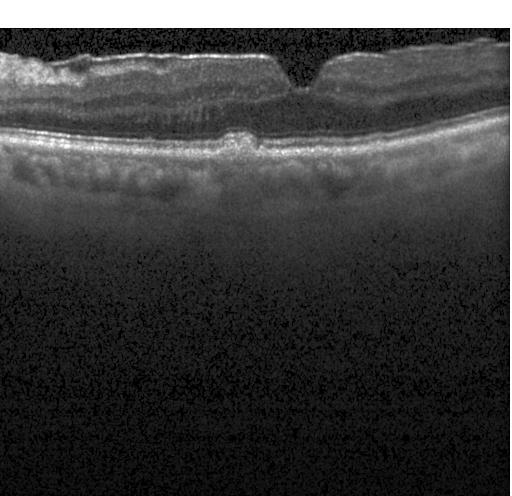
Macular OCT demonstrating sub-RPE drusenoid deposits.